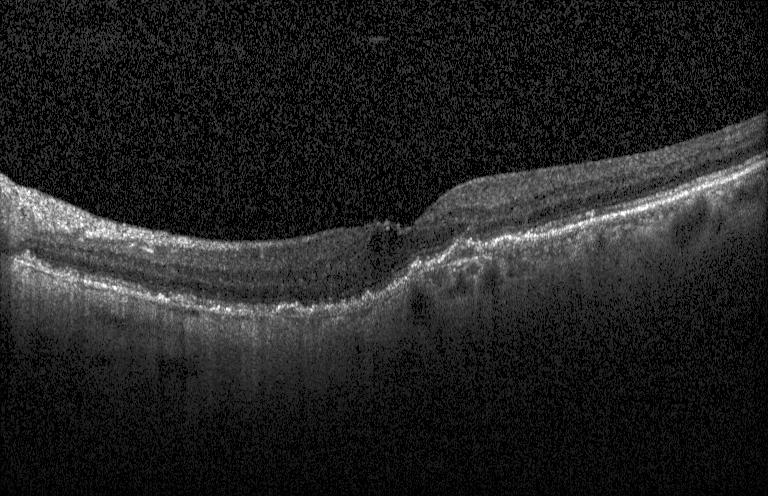 Optical coherence tomography B-scan. Macular OCT: choroidal neovascularization.